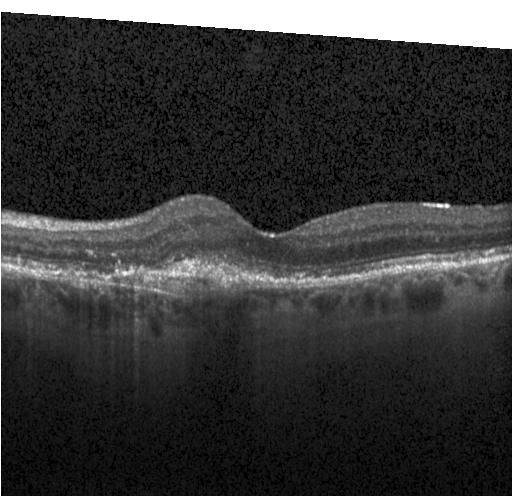
Optical coherence tomography scan. Fovea-centered
Finding: choroidal neovascularization (CNV).